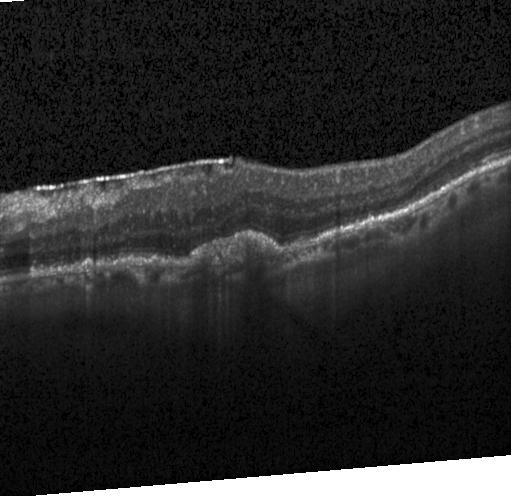
Retinal OCT B-scan. Fovea-centered. Spectral-domain OCT. Dx: choroidal neovascularization (CNV).